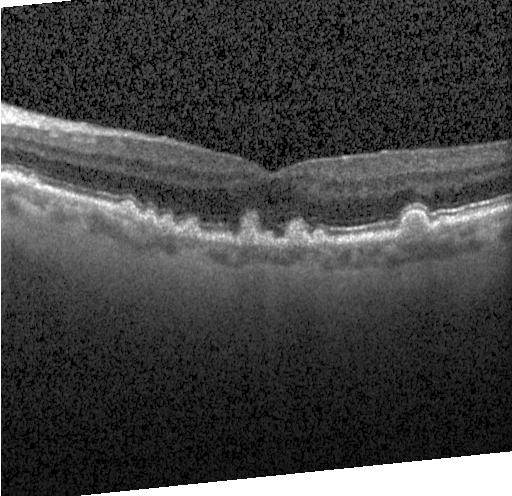 Centered on the fovea. OCT B-scan — Impression: multiple drusen.